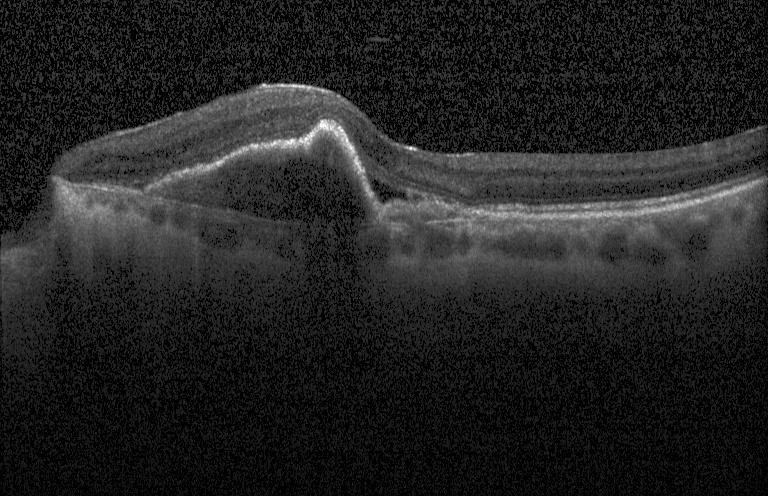

OCT line scan · horizontal scan through the fovea.
A choroidal neovascular membrane.